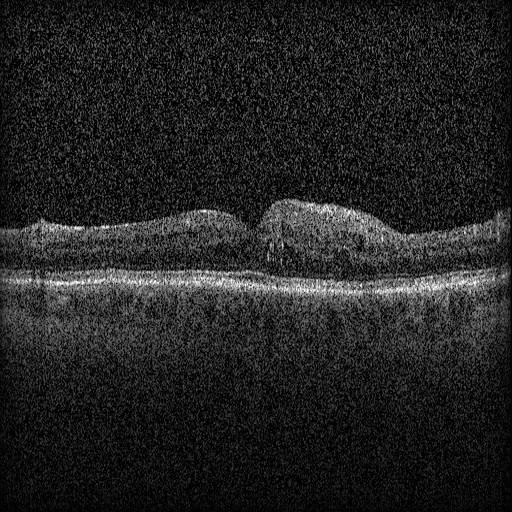
Fovea-centered. Optical coherence tomography scan. Acquired on a Heidelberg Spectralis
Diabetic macular edema (DME).